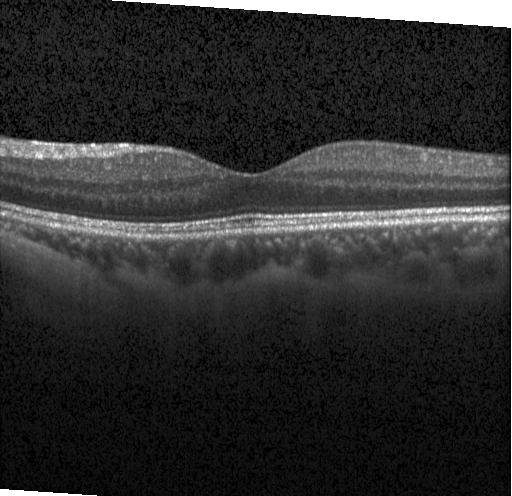

OCT B-scan; fovea-centered
Diagnosis: no evidence of choroidal neovascularization, diabetic macular edema, or drusen.